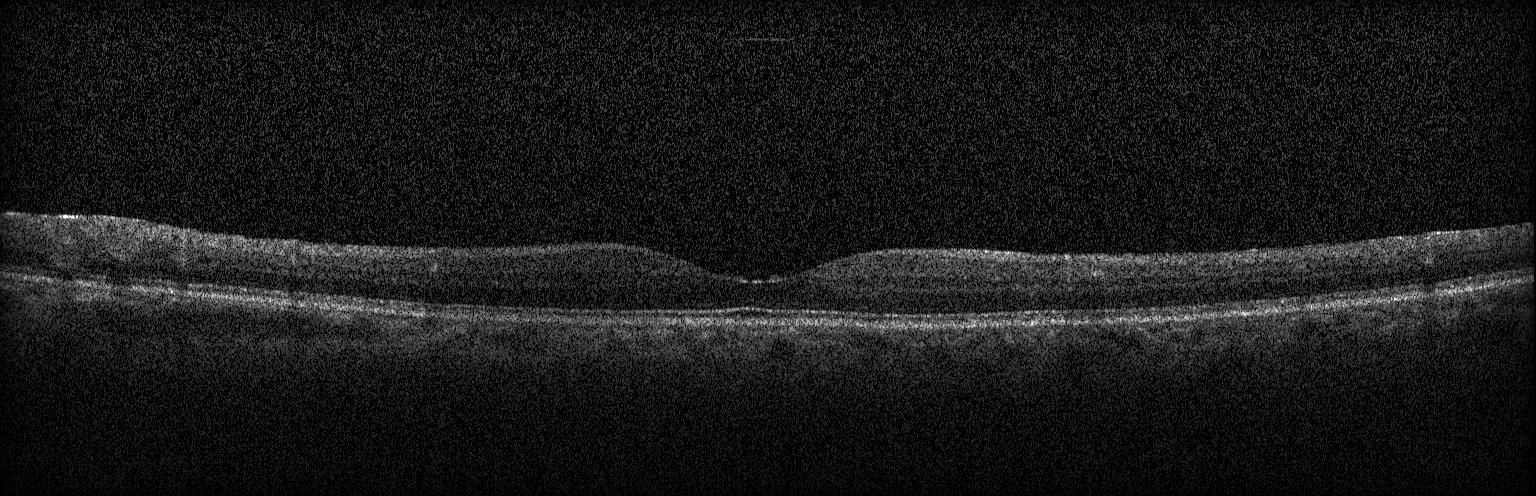
Horizontal scan through the fovea; spectral-domain optical coherence tomography; retinal OCT cross-section; Heidelberg Spectralis OCT system
Diagnosis: no choroidal neovascularization, diabetic macular edema, or drusen.